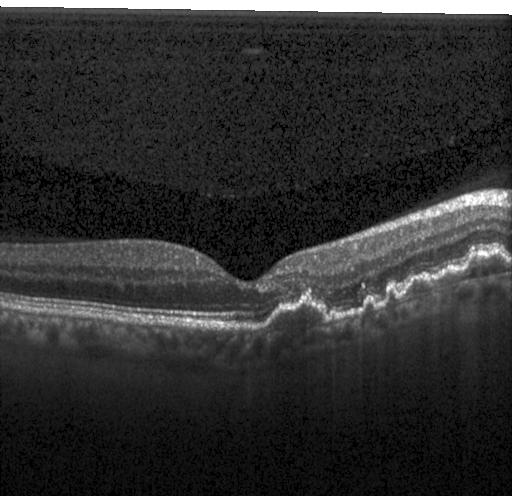
Retinal OCT B-scan; spectral-domain OCT; Heidelberg Spectralis. OCT finding: choroidal neovascularization.